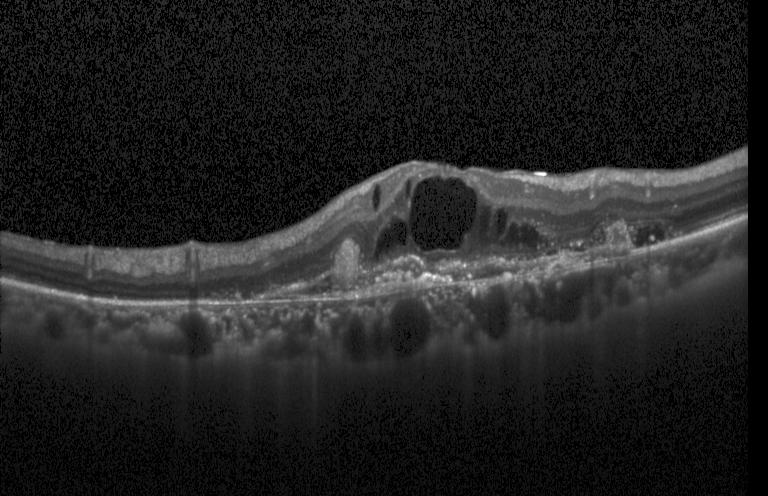 Macular OCT demonstrating a choroidal neovascular membrane.